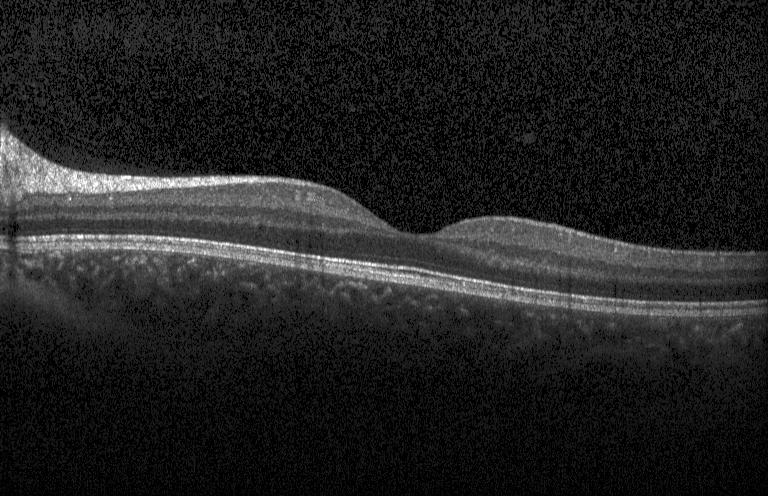

Retinal OCT cross-section. Through the macula. SD-OCT.
Dx: neither choroidal neovascularization, diabetic macular edema, nor drusen.